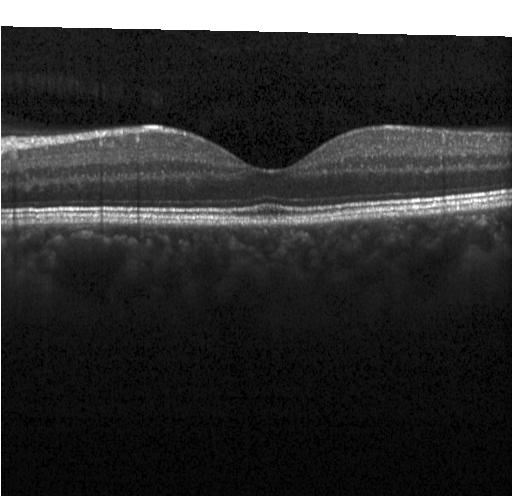
This B-scan demonstrates neither CNV, DME, nor drusen.